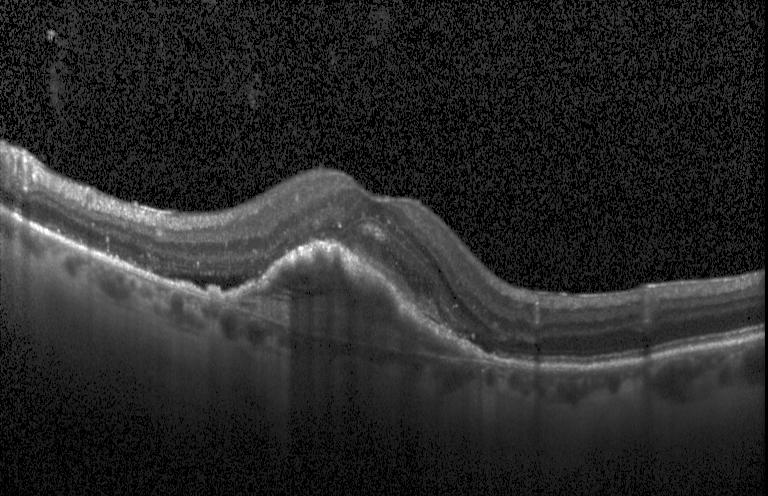

Macular OCT demonstrating choroidal neovascularization (CNV).